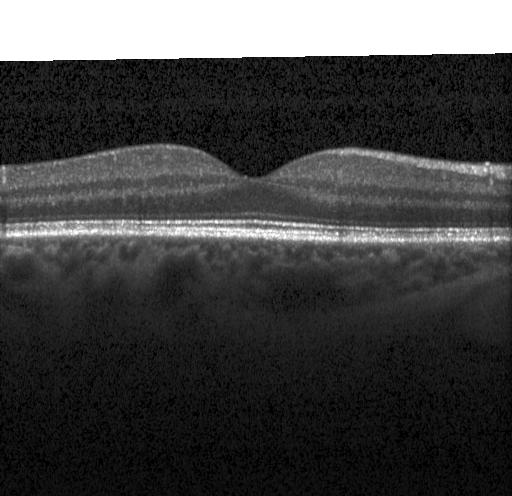
Macular OCT: neither choroidal neovascularization, diabetic macular edema, nor drusen.